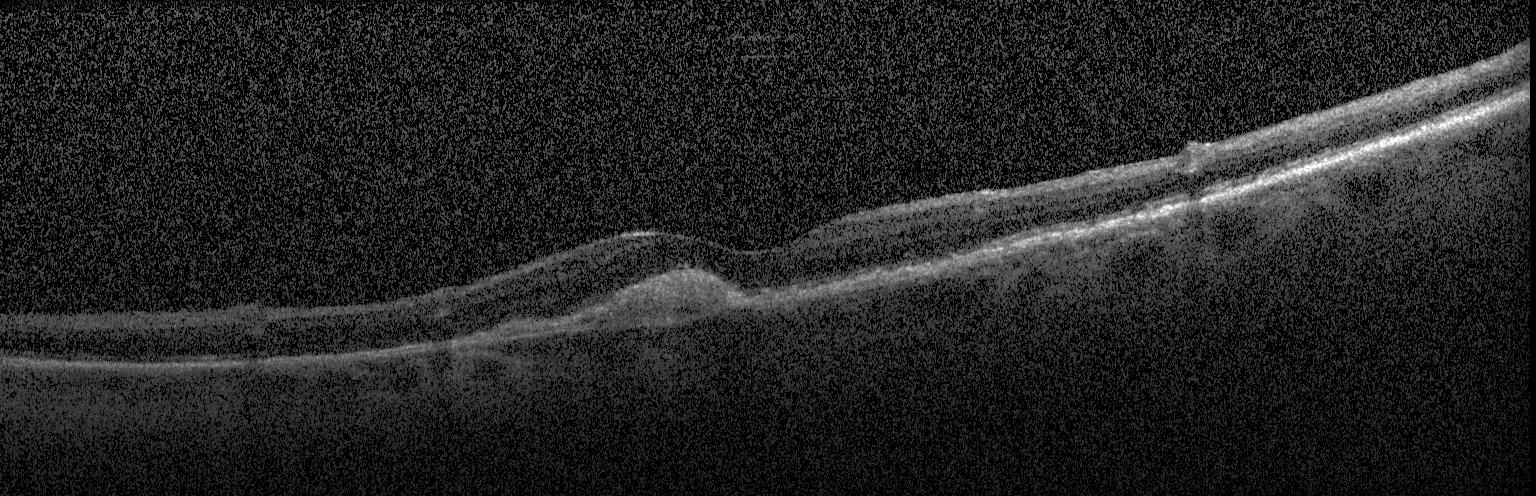
Through the macula; spectral-domain OCT; optical coherence tomography B-scan
Dx: a choroidal neovascular membrane.